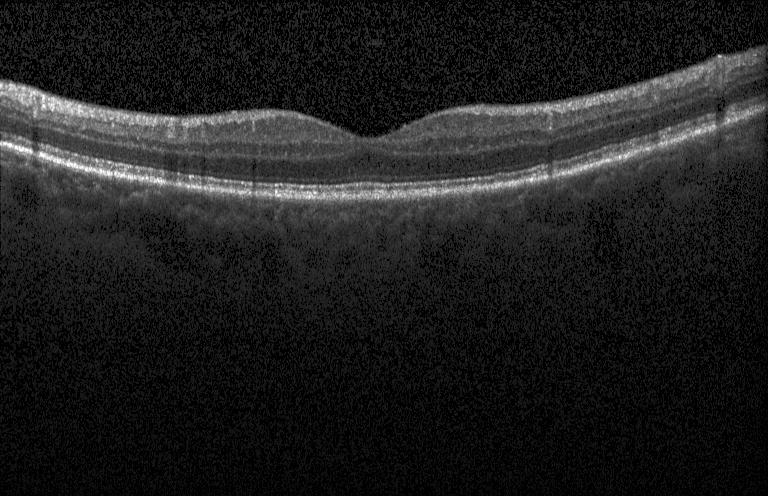

Horizontal scan through the fovea. OCT line scan
Diagnosis: no evidence of choroidal neovascularization, diabetic macular edema, or drusen.